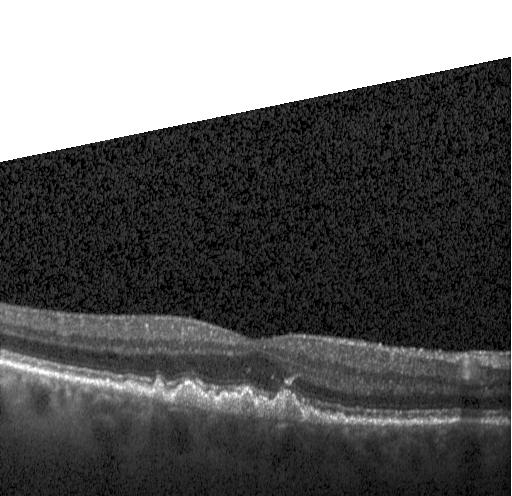
Spectral-domain OCT B-scan: drusen.